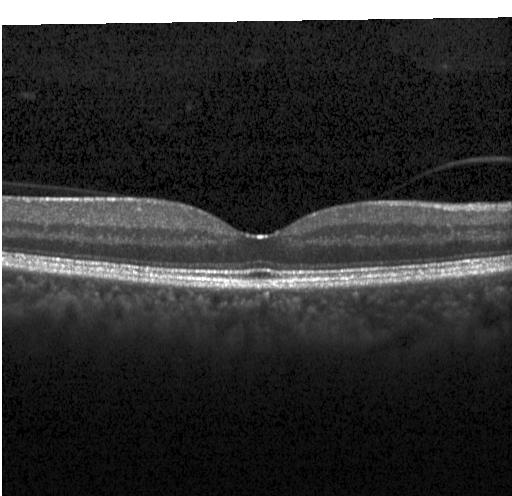

Spectral-domain optical coherence tomography. Horizontal scan through the fovea. Acquired on a Heidelberg Spectralis. Optical coherence tomography scan.
No evidence of CNV, DME, or drusen.